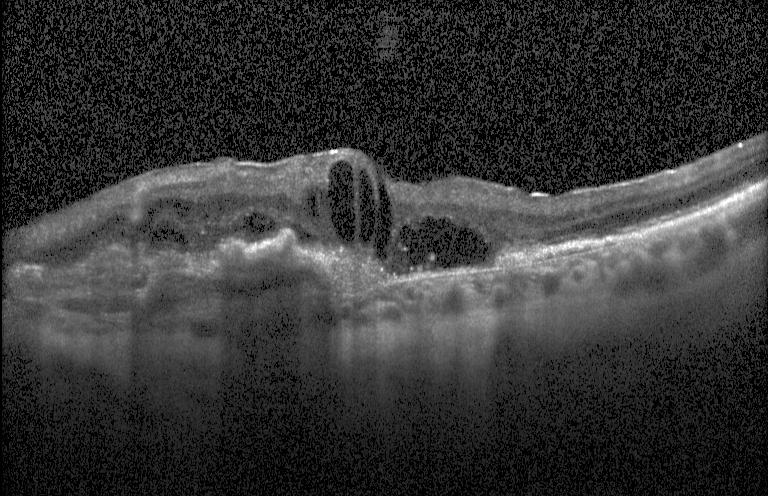 OCT B-scan. Impression: choroidal neovascularization (CNV).